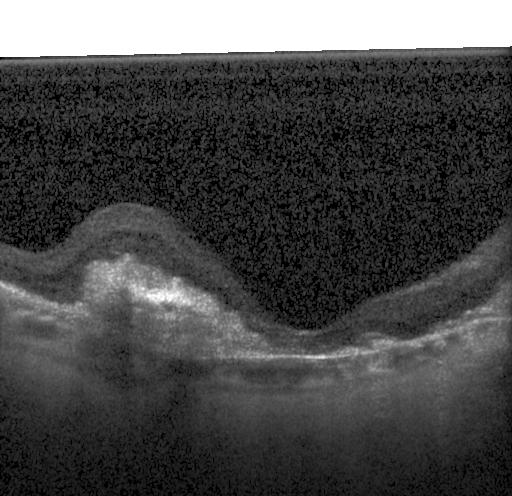

SD-OCT. Through the macula. OCT B-scan. Finding: choroidal neovascularization (CNV).